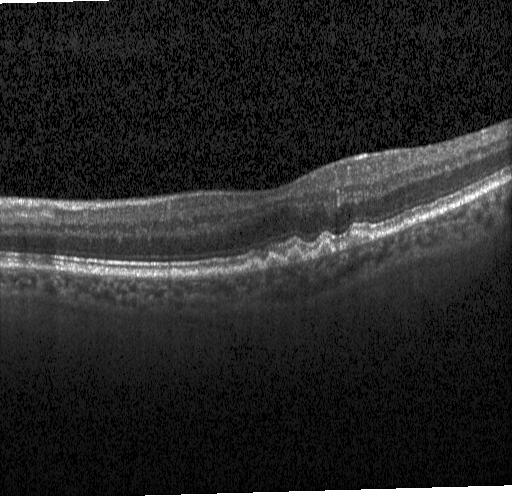

Heidelberg Spectralis OCT system. Horizontal scan through the fovea. Optical coherence tomography B-scan.
Finding: sub-RPE drusenoid deposits.